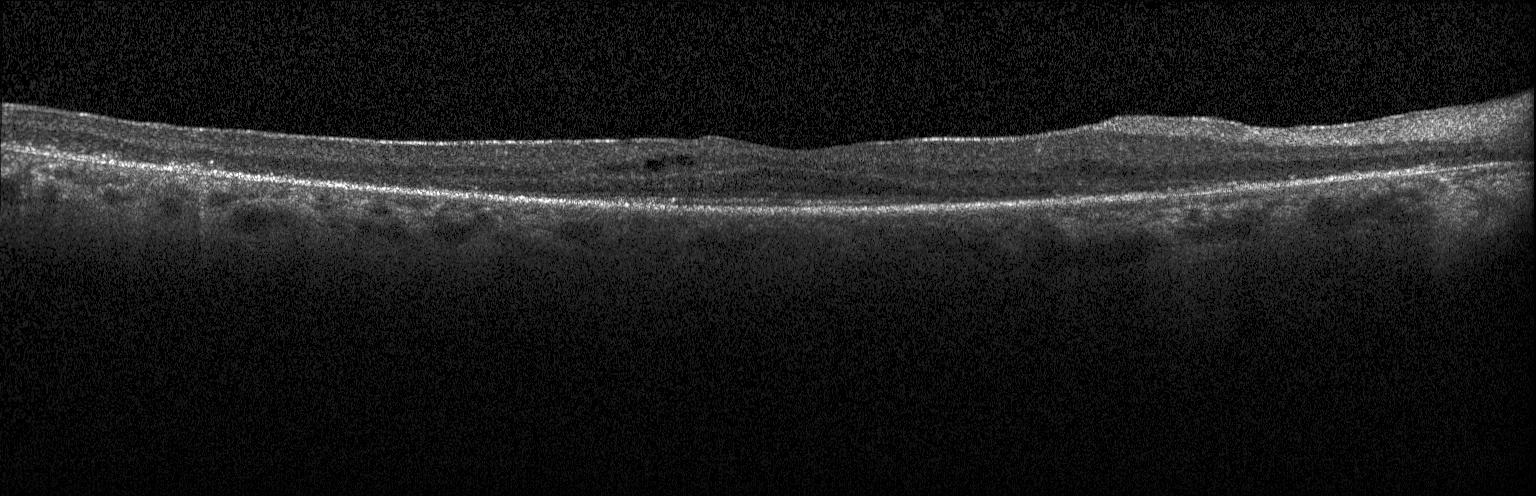 Macular scan. Spectral-domain optical coherence tomography. Retinal OCT cross-section. Heidelberg Spectralis. Impression: diabetic macular edema.